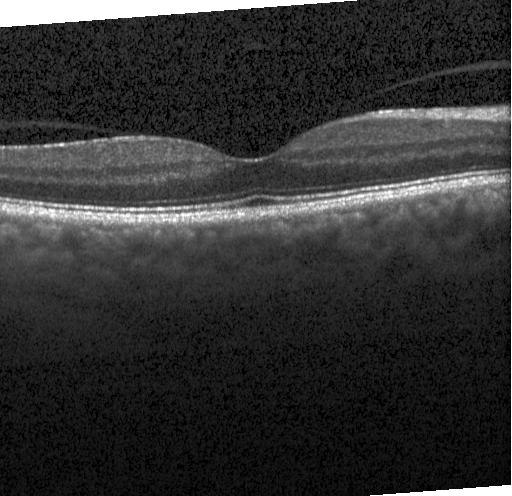 Impression: no choroidal neovascularization, diabetic macular edema, or drusen.